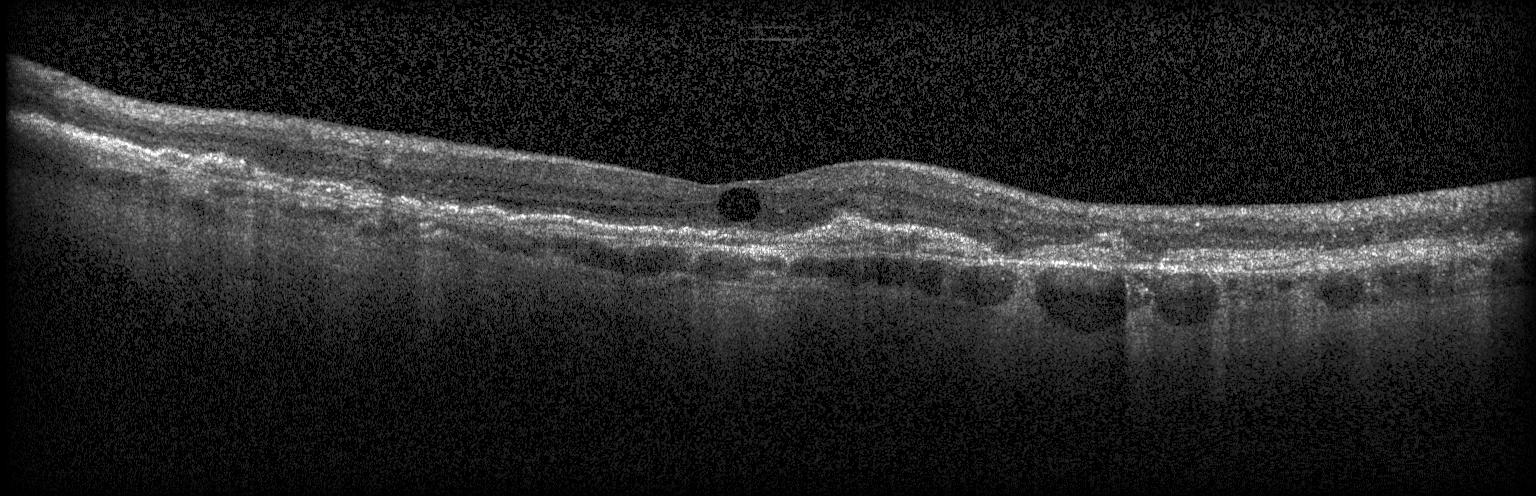
OCT scan showing a choroidal neovascular membrane.